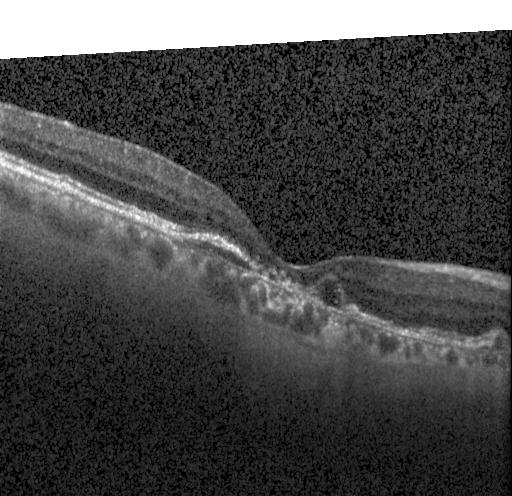
Optical coherence tomography B-scan. Macular scan. Diagnosis: CNV.